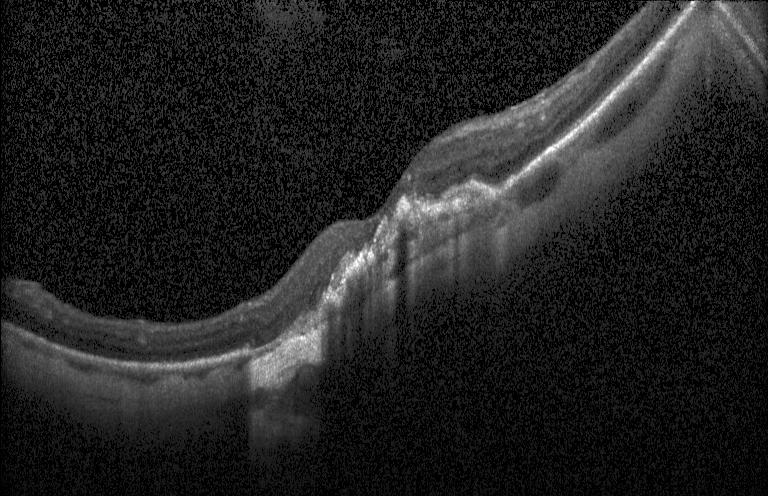

Retinal OCT B-scan · spectral-domain OCT · horizontal scan through the fovea · Heidelberg Spectralis — Macular OCT: choroidal neovascularization.